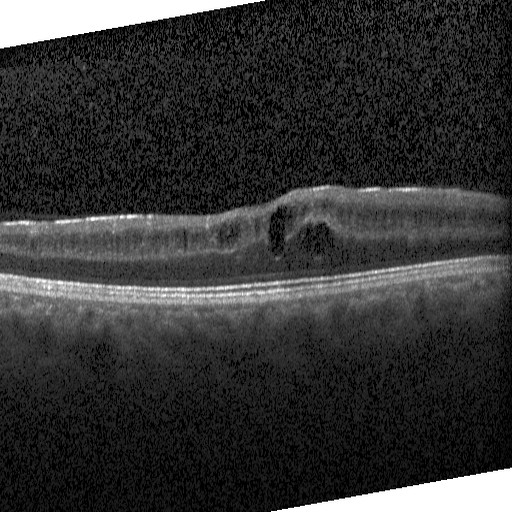

Finding: DME.